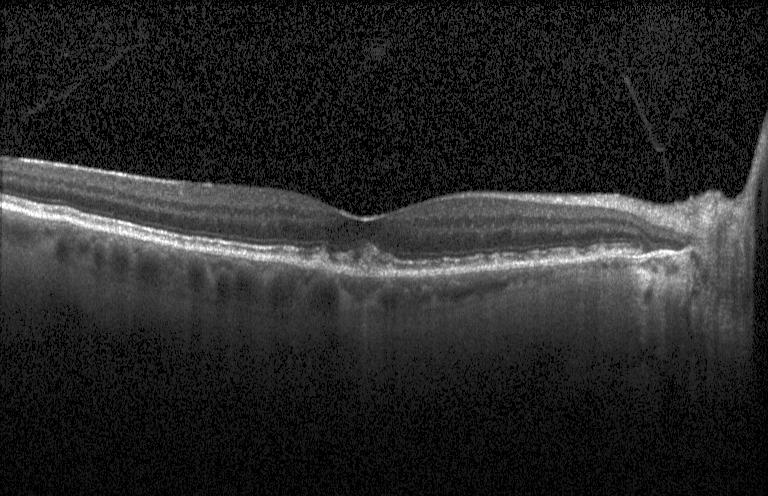 Impression: sub-RPE drusenoid deposits.